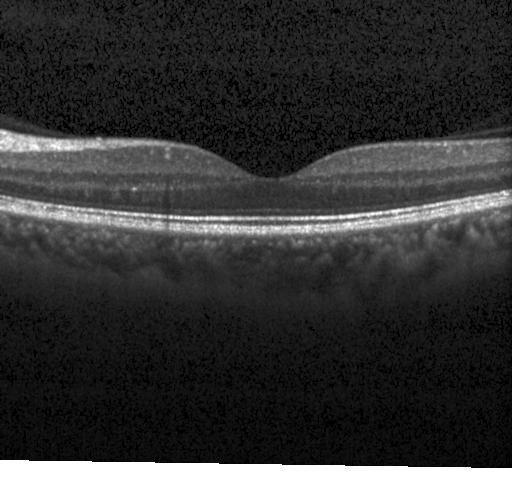 Instrument: Heidelberg Spectralis. Spectral-domain optical coherence tomography. Through the macula. OCT B-scan.
Diagnosis: no evidence of choroidal neovascularization, diabetic macular edema, or drusen.